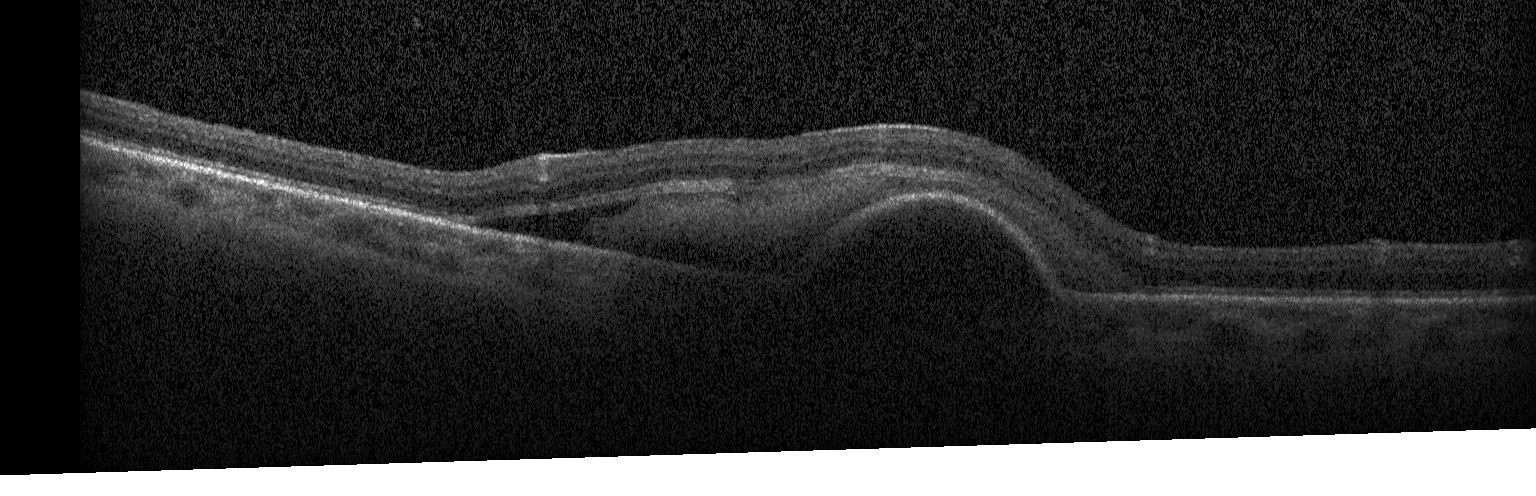

Retinal OCT B-scan, instrument: Heidelberg Spectralis, SD-OCT, centered on the fovea — Assessment: choroidal neovascularization.